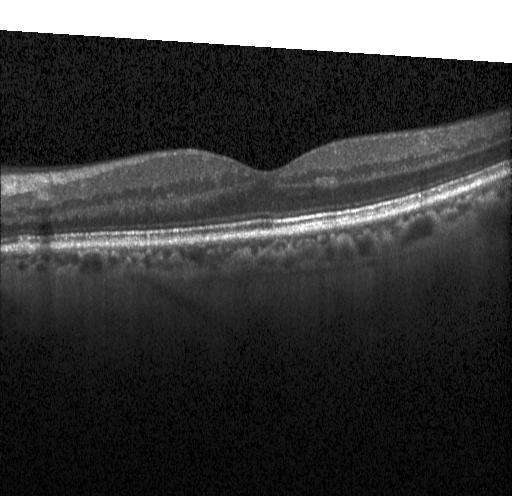

Macular OCT: no CNV, DME, or drusen.